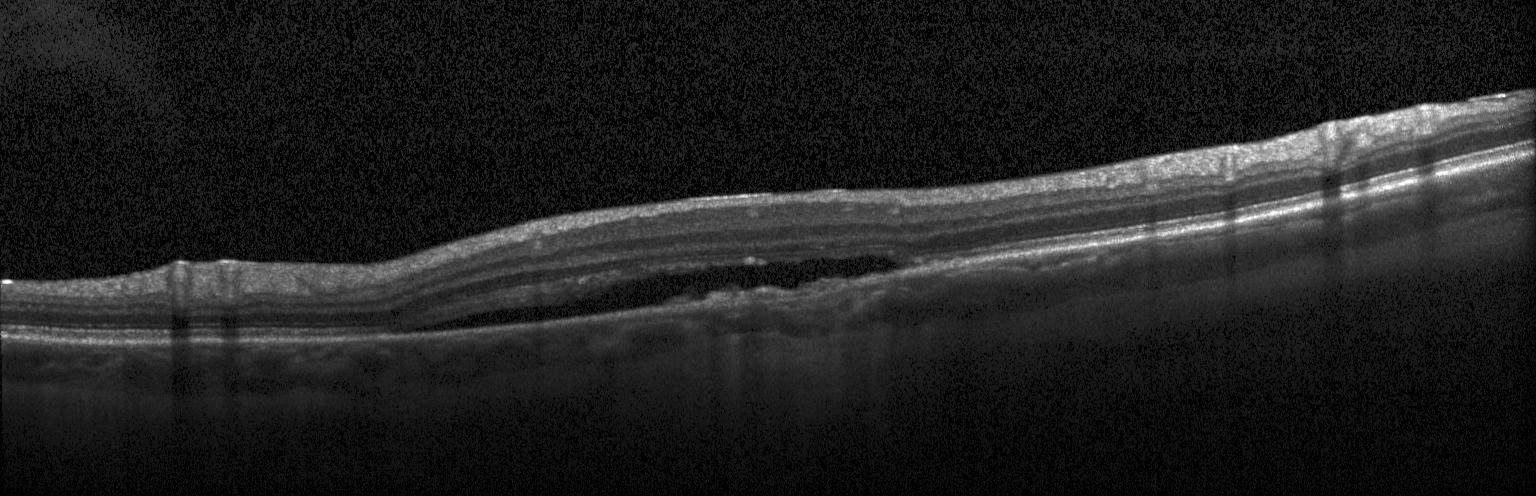 Heidelberg Spectralis; optical coherence tomography B-scan. Diagnosis: a choroidal neovascular membrane.